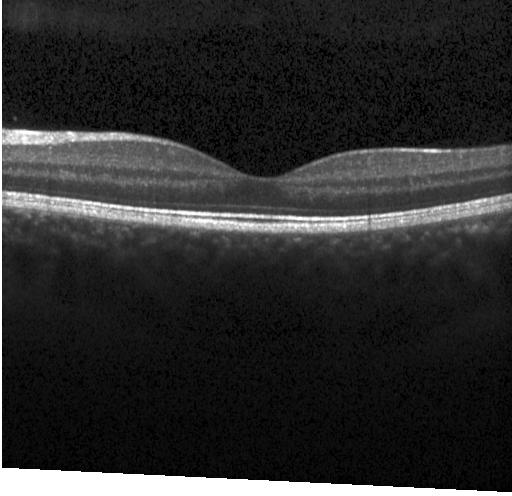 SD-OCT, retinal OCT B-scan, Heidelberg Spectralis OCT system.
This B-scan demonstrates neither CNV, DME, nor drusen.